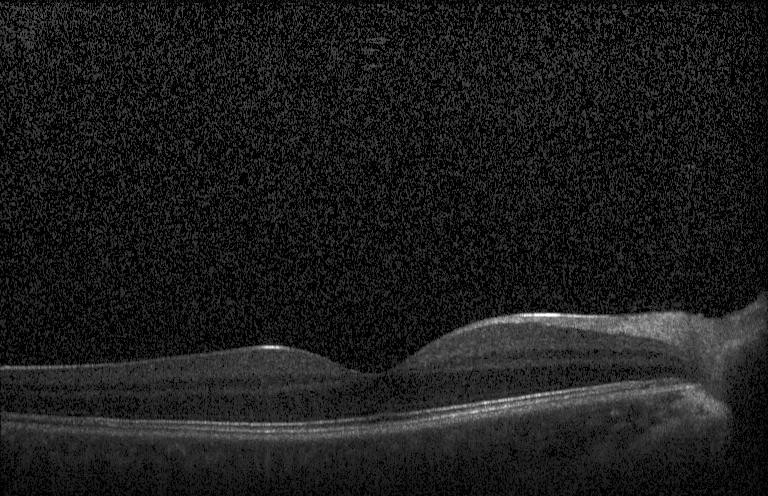
Macular OCT demonstrating no evidence of choroidal neovascularization, diabetic macular edema, or drusen.